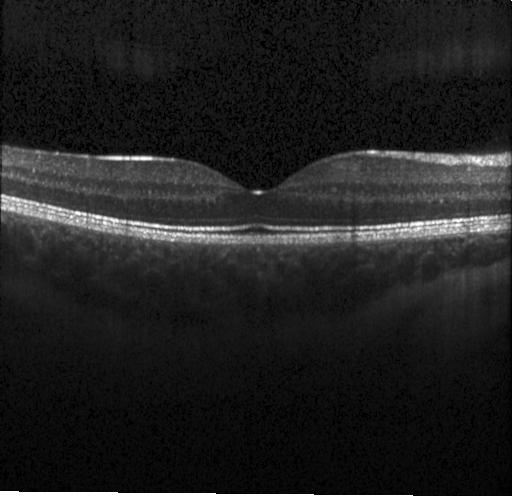 Heidelberg Spectralis OCT system, through the macula, OCT line scan, spectral-domain optical coherence tomography. Diagnosis: no CNV, DME, or drusen.